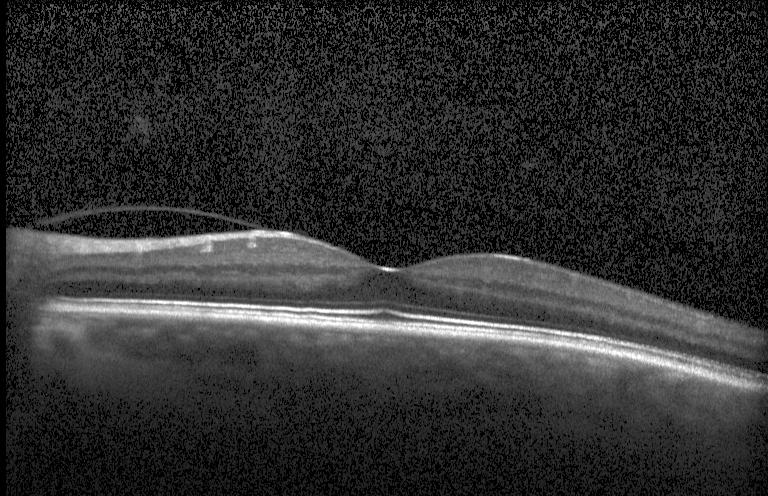
Macular OCT demonstrating neither CNV, DME, nor drusen.